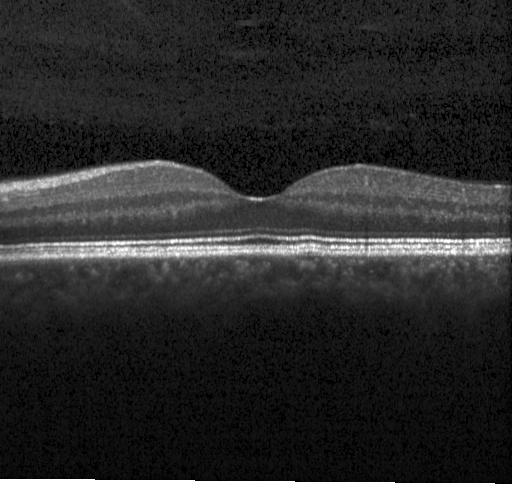 SD-OCT, OCT B-scan, Heidelberg Spectralis OCT system — Macular OCT: neither choroidal neovascularization, diabetic macular edema, nor drusen.